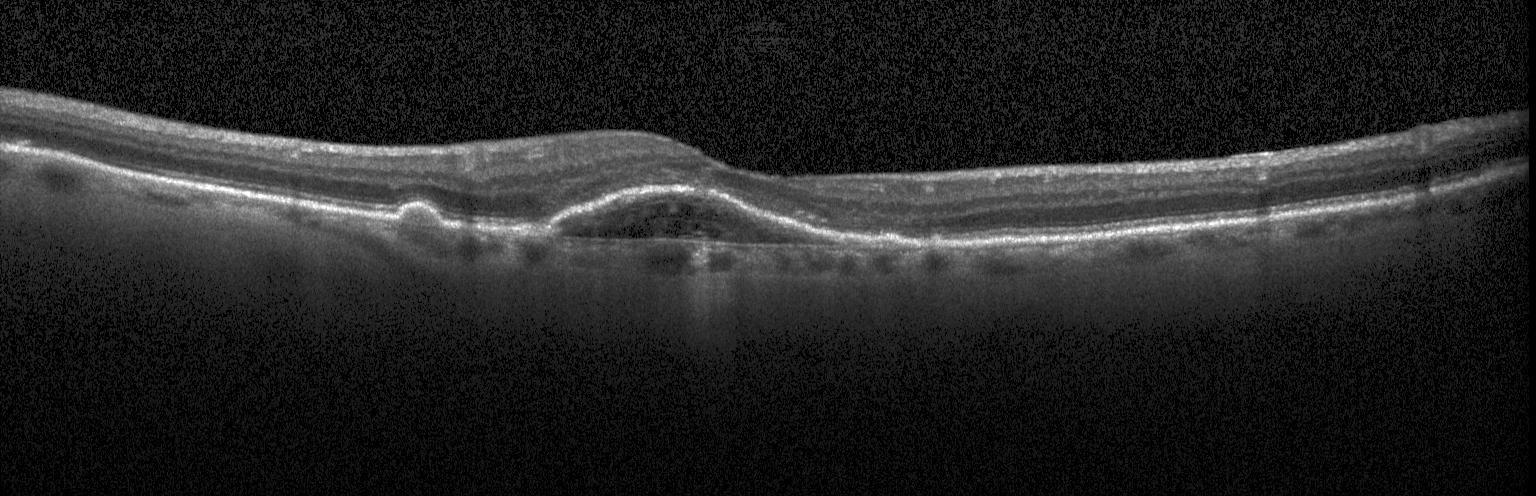
OCT line scan — A choroidal neovascular membrane.